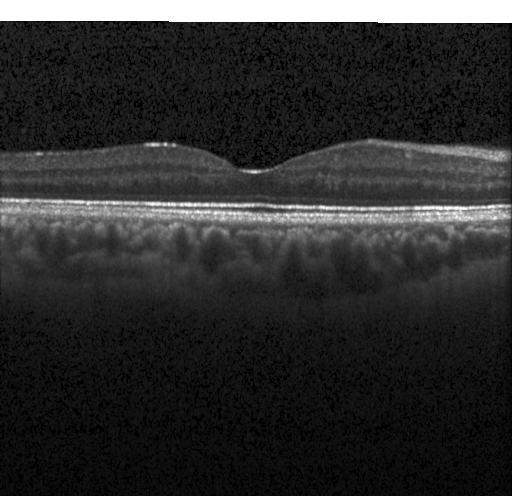

Macular scan; optical coherence tomography B-scan.
Assessment: neither CNV, DME, nor drusen.